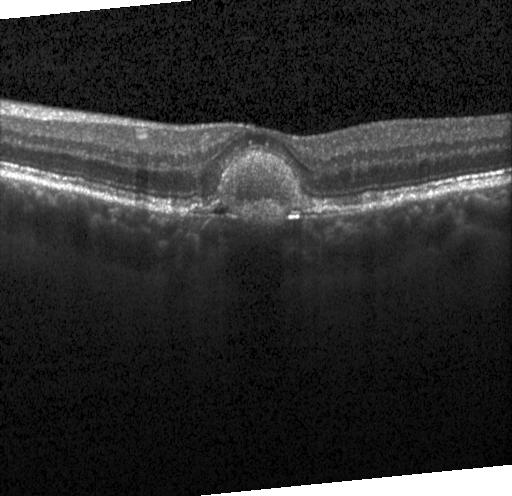

Finding: CNV.